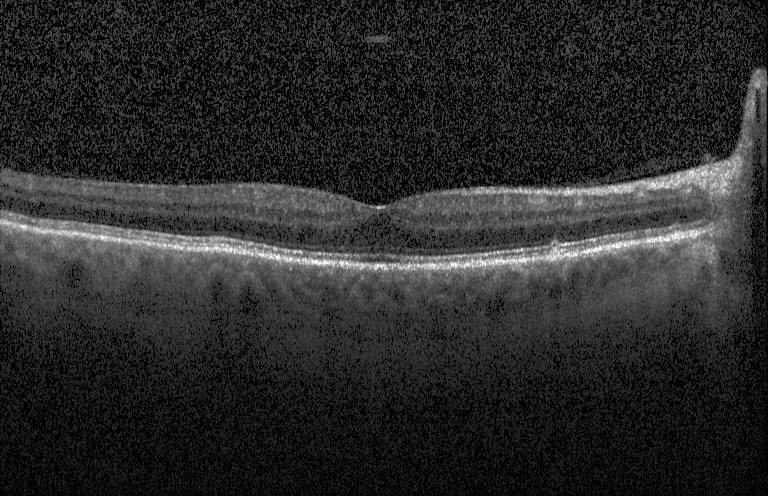 Retinal OCT cross-section, Heidelberg Spectralis, centered on the fovea, SD-OCT
The scan shows no evidence of choroidal neovascularization, diabetic macular edema, or drusen.